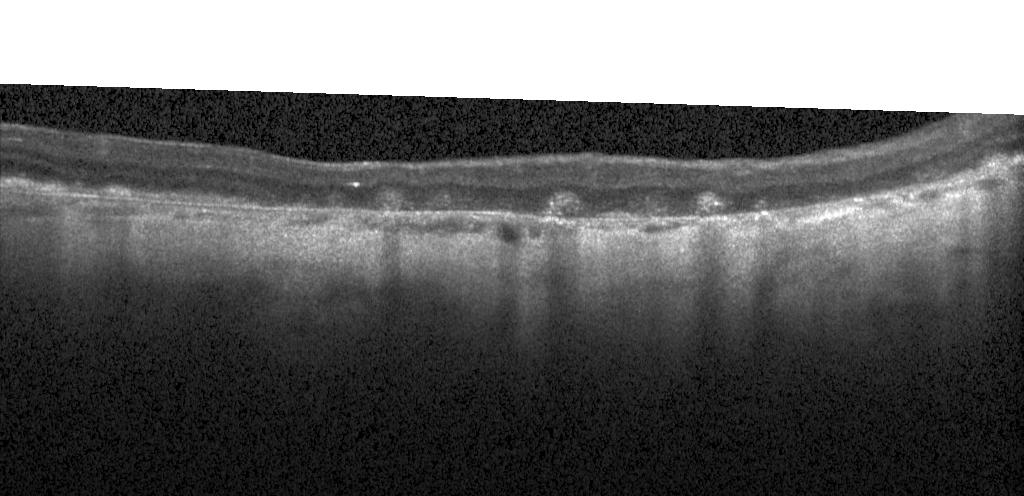 Impression: no evidence of choroidal neovascularization, diabetic macular edema, or drusen.